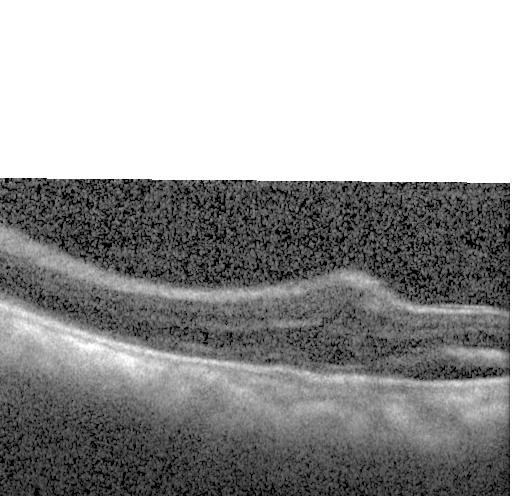 SD-OCT, optical coherence tomography B-scan, macular scan
Diagnosis: choroidal neovascularization (CNV).